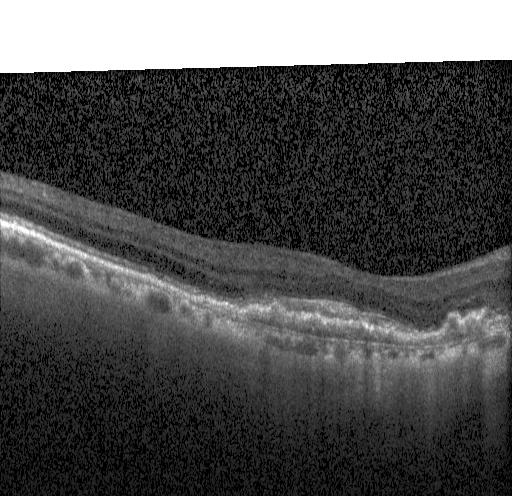
Centered on the fovea; retinal OCT B-scan; Heidelberg Spectralis. This B-scan demonstrates a choroidal neovascular membrane.